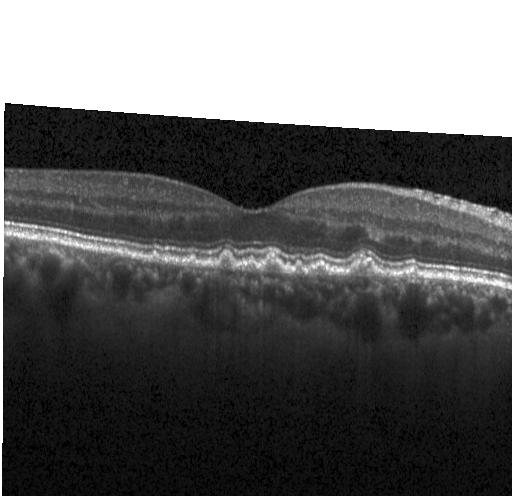
OCT B-scan. Sub-RPE drusenoid deposits.